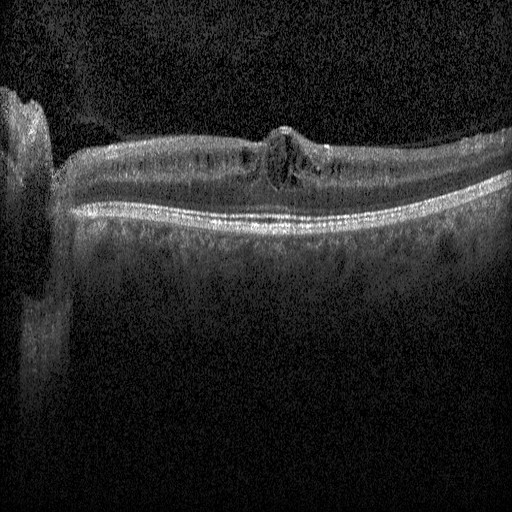
Instrument: Heidelberg Spectralis, macular scan, OCT B-scan, SD-OCT — Diagnosis: diabetic macular edema.